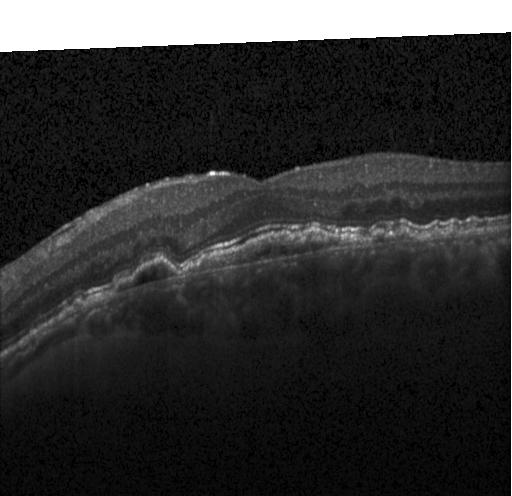 Retinal OCT cross-section showing choroidal neovascularization.